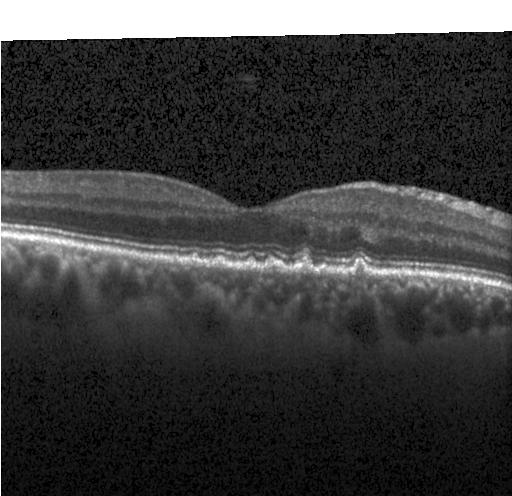
Centered on the fovea · OCT B-scan. Macular OCT: drusen.